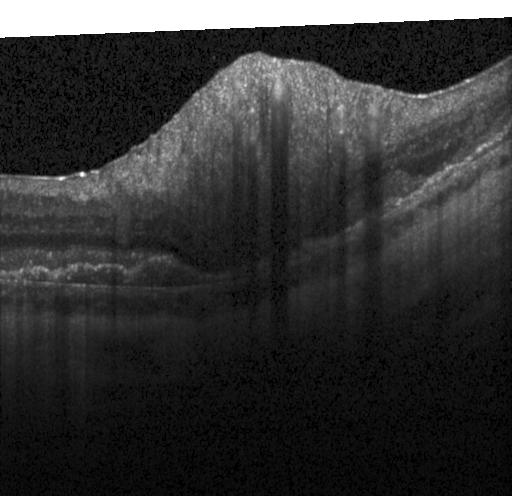 Macular OCT: choroidal neovascularization.